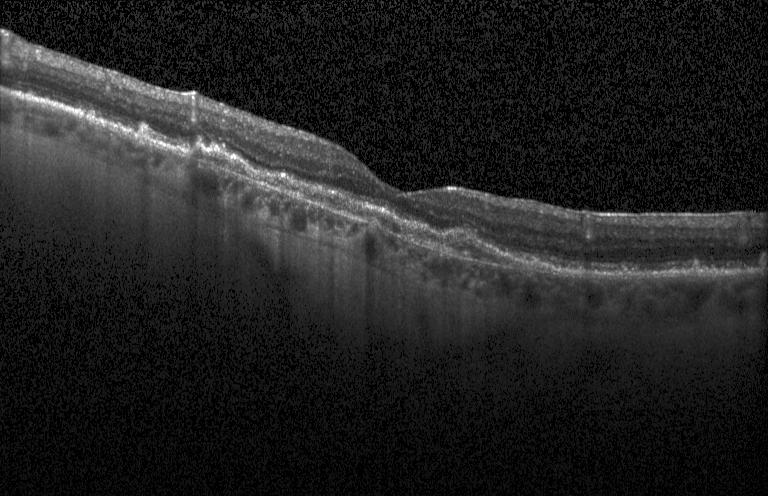 OCT B-scan. The scan shows a choroidal neovascular membrane.